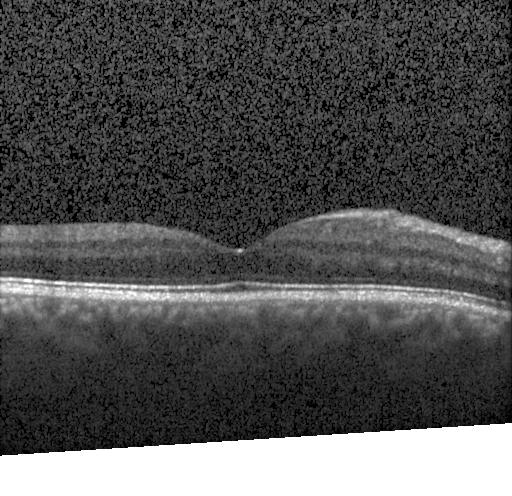 OCT finding: no evidence of CNV, DME, or drusen.